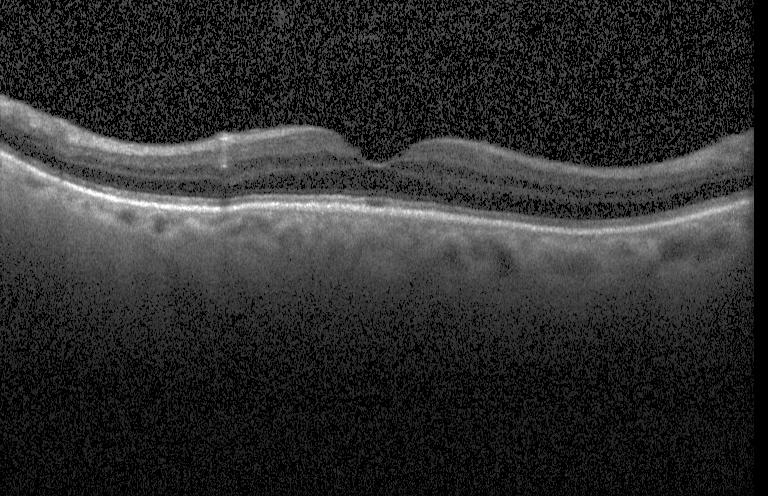
SD-OCT; macular scan; retinal OCT cross-section. This B-scan demonstrates neither choroidal neovascularization, diabetic macular edema, nor drusen.